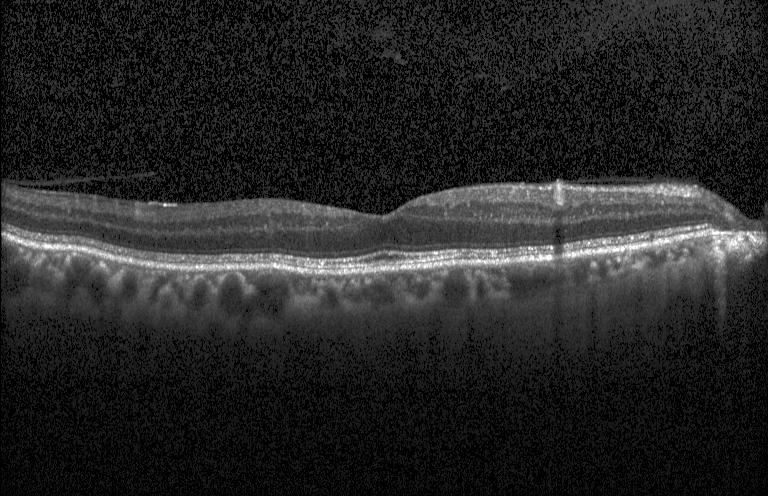 Centered on the fovea, Heidelberg Spectralis OCT system, optical coherence tomography B-scan, SD-OCT — Diagnosis: neither choroidal neovascularization, diabetic macular edema, nor drusen.